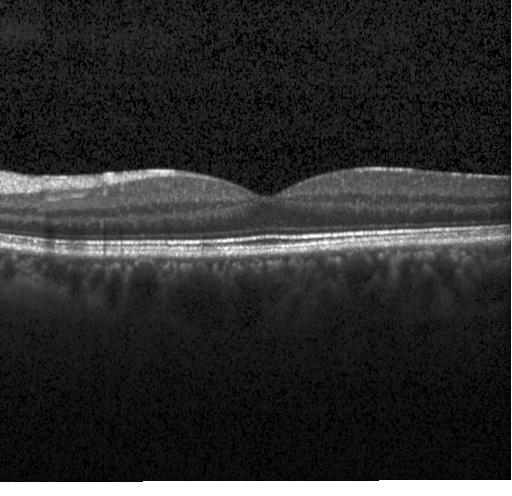

Optical coherence tomography scan, spectral-domain optical coherence tomography, Heidelberg Spectralis. Diagnosis: no CNV, DME, or drusen.